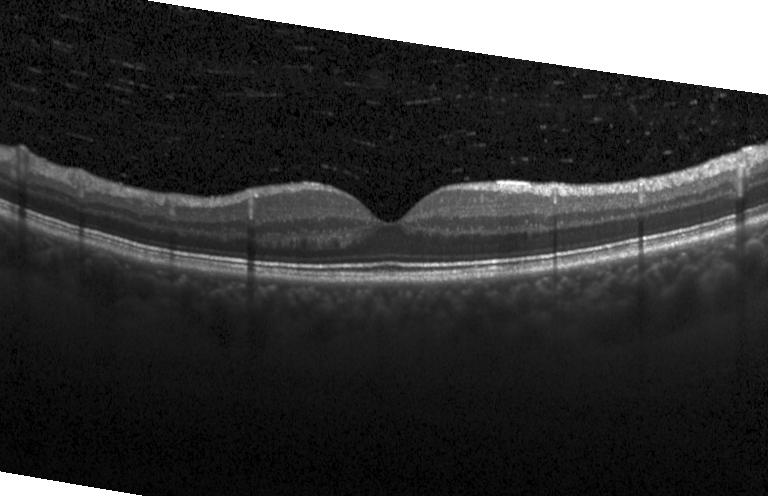

Retinal OCT cross-section, spectral-domain optical coherence tomography.
This B-scan demonstrates neither choroidal neovascularization, diabetic macular edema, nor drusen.